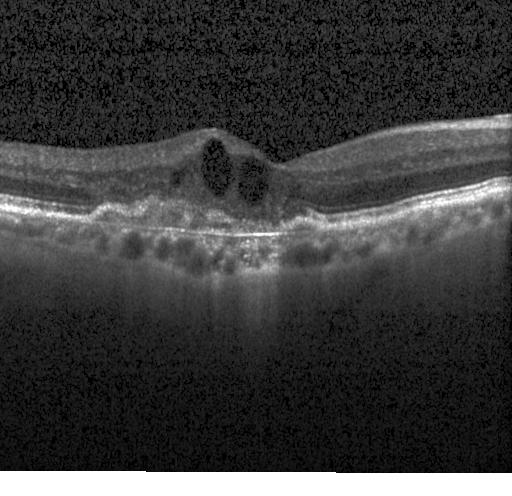 Optical coherence tomography B-scan, horizontal scan through the fovea, acquired on a Heidelberg Spectralis. The scan shows CNV.